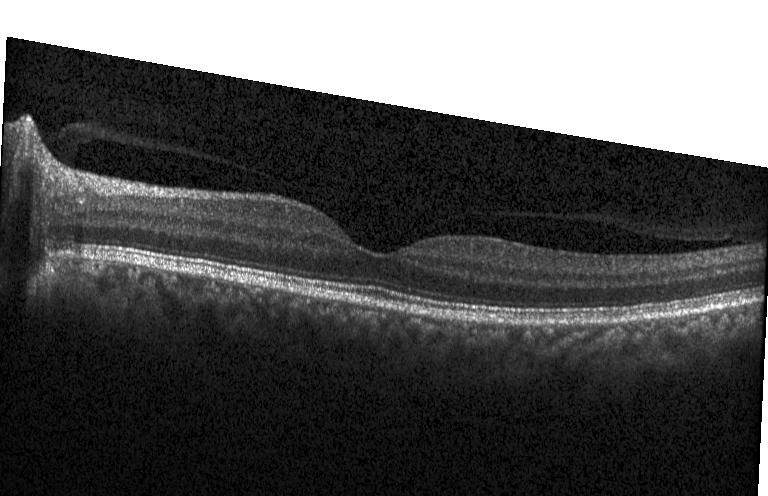
Macular scan. Optical coherence tomography B-scan
Impression: no choroidal neovascularization, diabetic macular edema, or drusen.